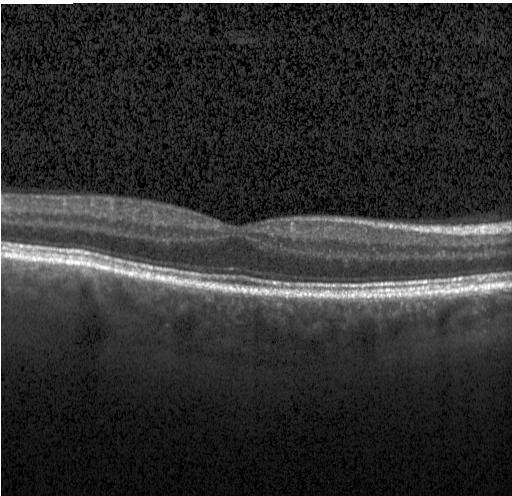

OCT line scan.
Impression: no evidence of choroidal neovascularization, diabetic macular edema, or drusen.